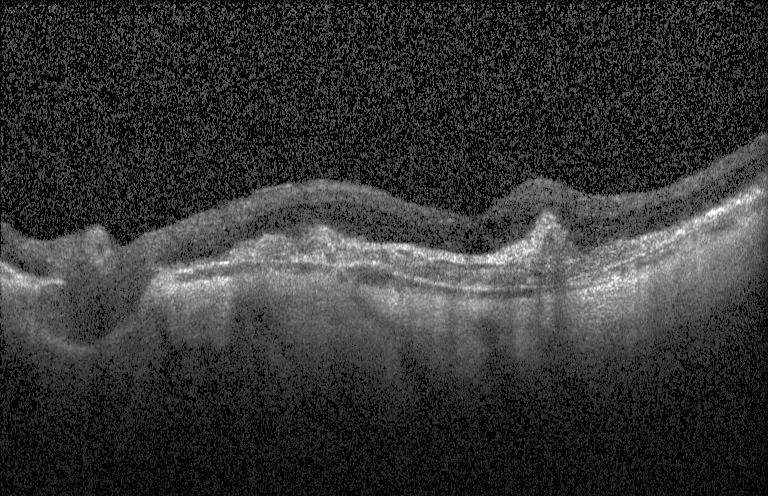 Spectral-domain OCT B-scan: a choroidal neovascular membrane.